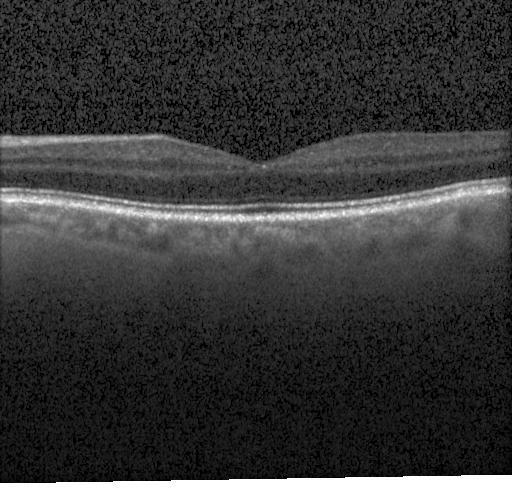
Finding: no evidence of choroidal neovascularization, diabetic macular edema, or drusen.